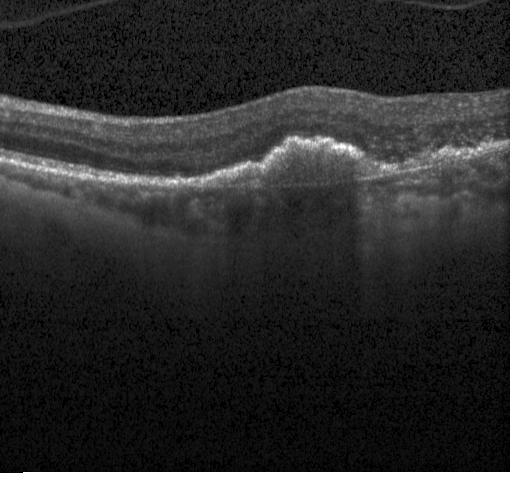 Retinal OCT cross-section showing a choroidal neovascular membrane.